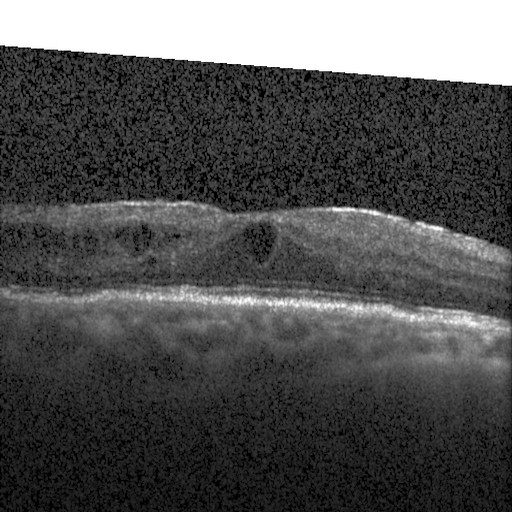 Fovea-centered. Optical coherence tomography scan. Acquired on a Heidelberg Spectralis. Spectral-domain OCT — Diagnosis: diabetic macular edema (DME).